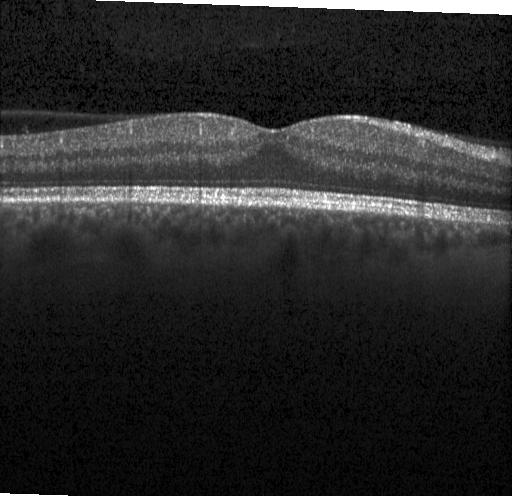
Through the macula; retinal OCT B-scan; spectral-domain optical coherence tomography; acquired on a Heidelberg Spectralis
Dx: neither choroidal neovascularization, diabetic macular edema, nor drusen.